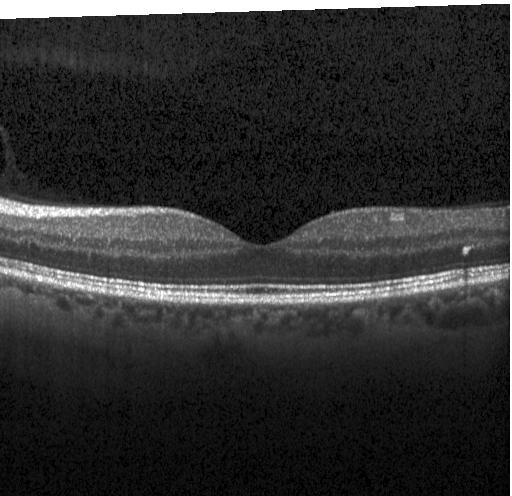

Instrument: Heidelberg Spectralis, spectral-domain OCT, retinal OCT cross-section.
Diagnosis: neither choroidal neovascularization, diabetic macular edema, nor drusen.